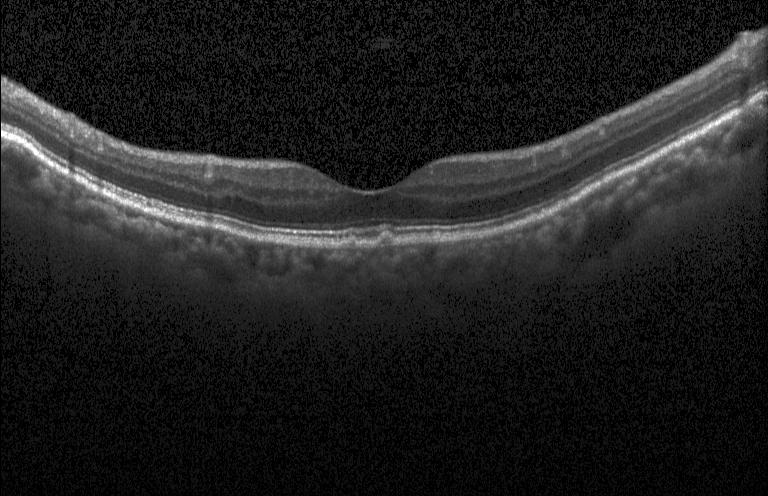
Horizontal scan through the fovea · instrument: Heidelberg Spectralis · SD-OCT · OCT B-scan — Impression: sub-RPE drusenoid deposits.